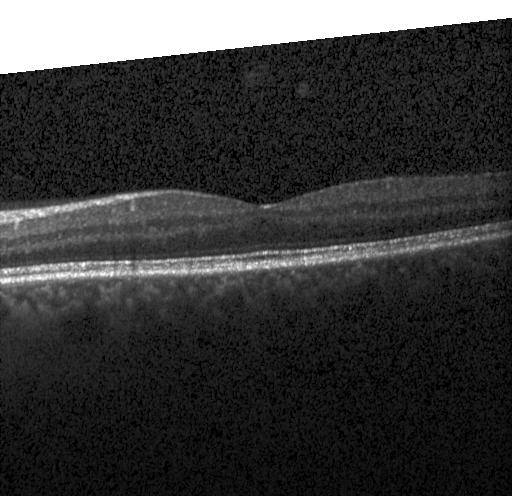 OCT line scan; Heidelberg Spectralis; macular scan; spectral-domain OCT — Macular OCT: no evidence of choroidal neovascularization, diabetic macular edema, or drusen.